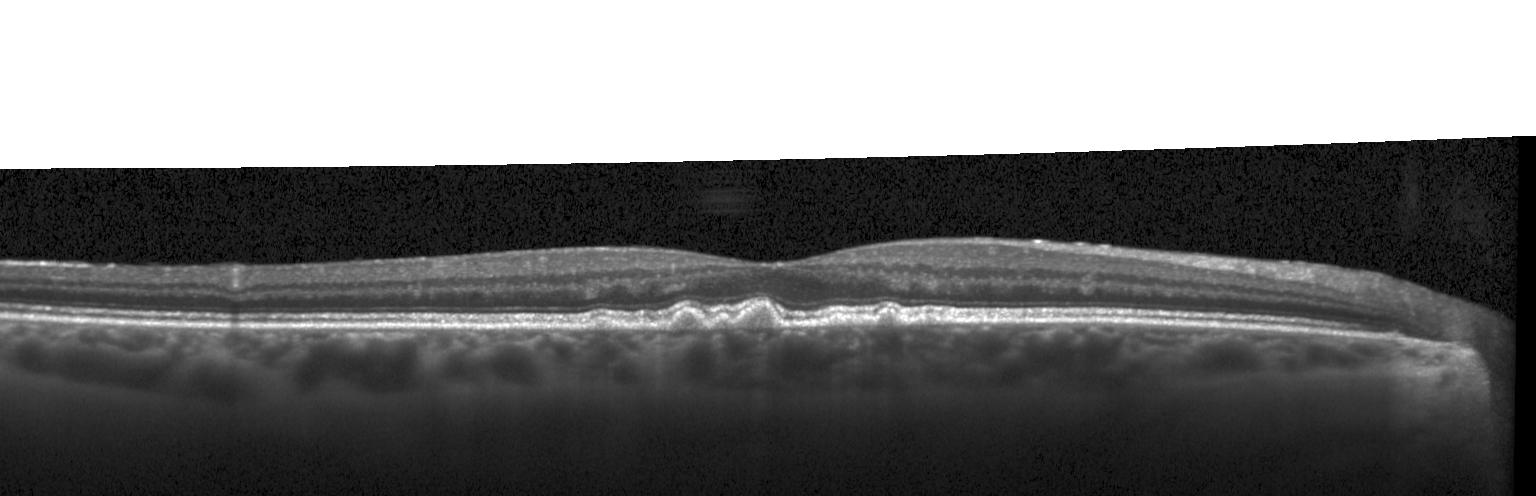
Retinal OCT B-scan · SD-OCT · Heidelberg Spectralis OCT system · centered on the fovea — Diagnosis: sub-RPE drusenoid deposits.